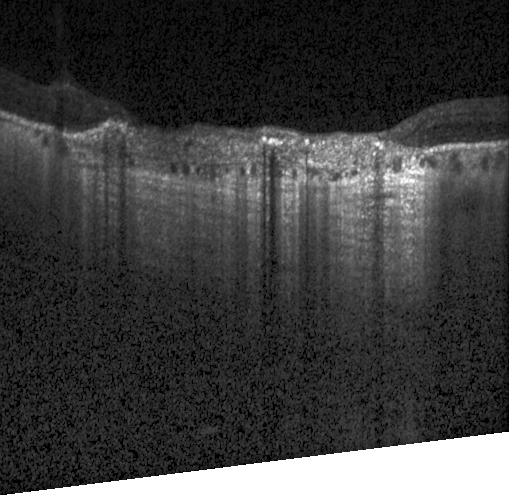 OCT scan showing a choroidal neovascular membrane.